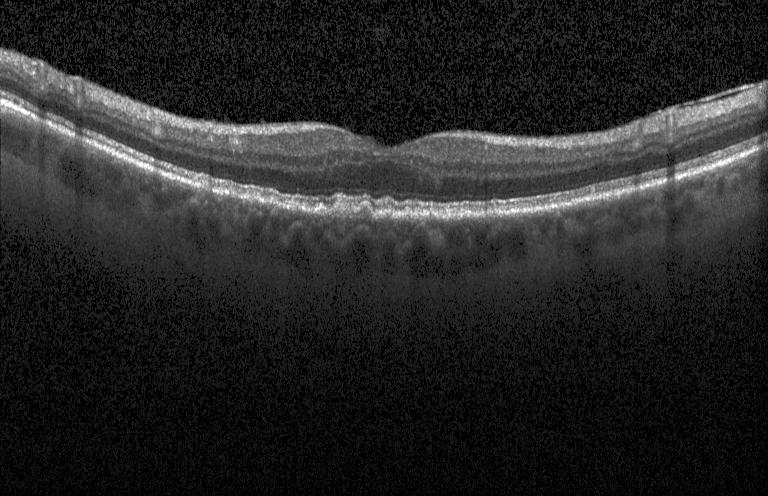 Finding: drusen.